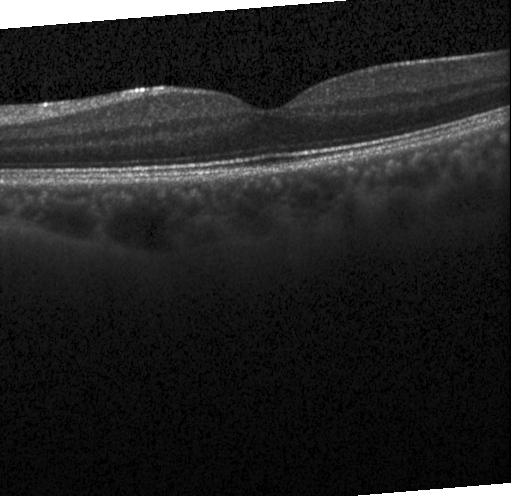 Through the macula · spectral-domain optical coherence tomography · Heidelberg Spectralis · OCT B-scan — Impression: no choroidal neovascularization, no diabetic macular edema, and no drusen.